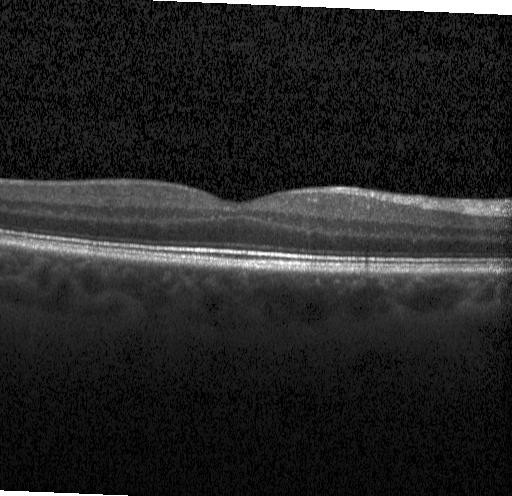 Spectral-domain OCT · through the macula · OCT B-scan · acquired on a Heidelberg Spectralis — The scan shows no evidence of CNV, DME, or drusen.